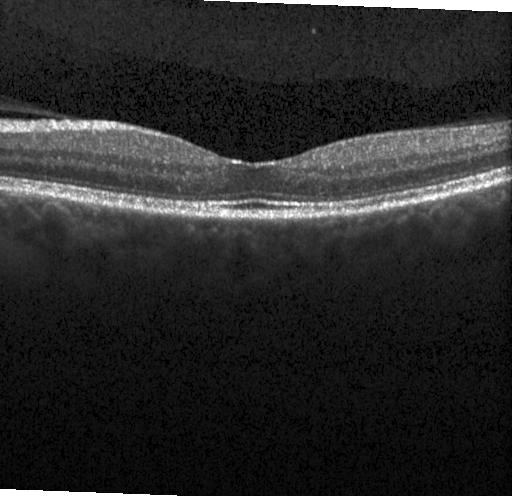 Optical coherence tomography scan · Heidelberg Spectralis — This B-scan demonstrates no choroidal neovascularization, no diabetic macular edema, and no drusen.